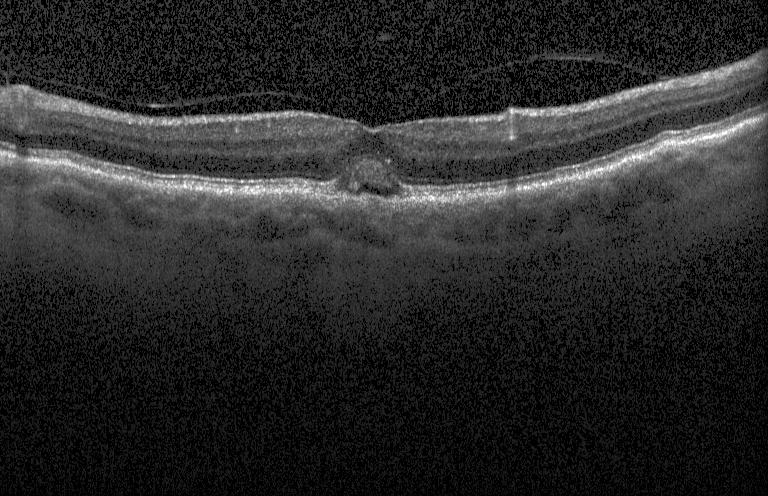 Optical coherence tomography B-scan. Through the macula. OCT finding: choroidal neovascularization.